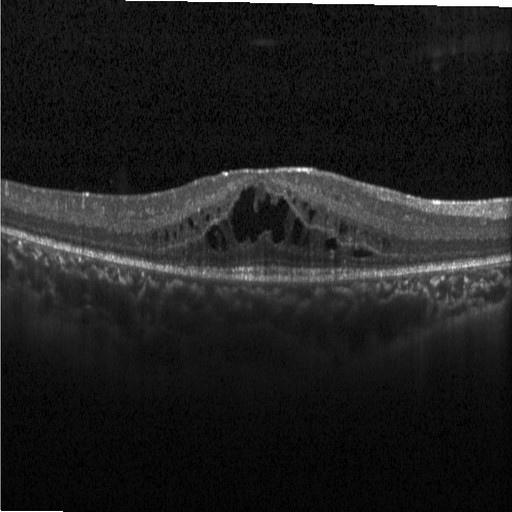

Macular OCT demonstrating diabetic macular edema (DME).